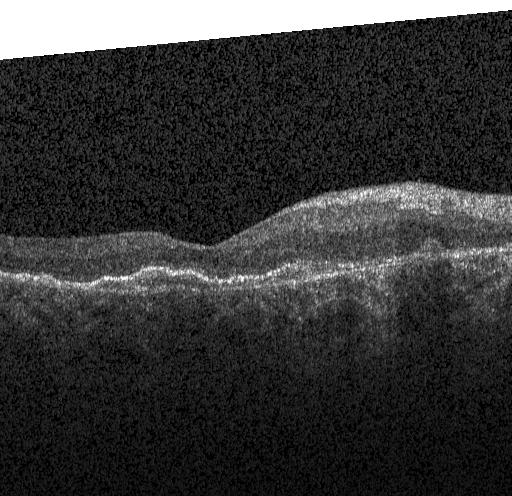

Instrument: Heidelberg Spectralis; optical coherence tomography B-scan; spectral-domain optical coherence tomography.
Macular OCT: choroidal neovascularization (CNV).